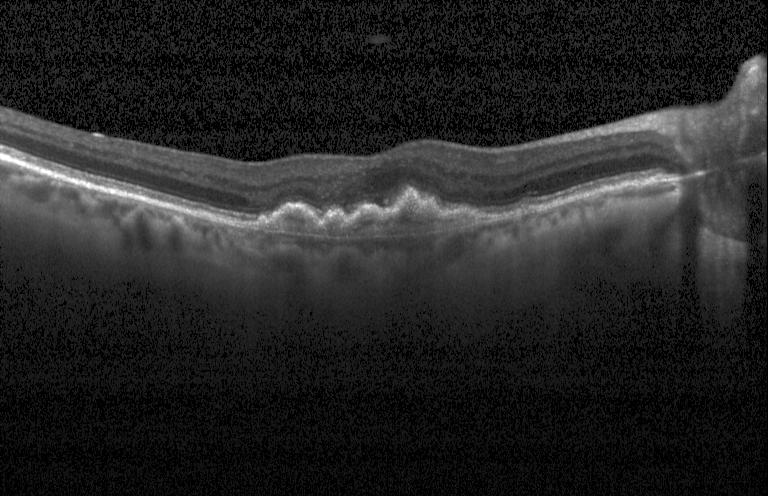
Retinal OCT B-scan, SD-OCT — Impression: choroidal neovascularization.